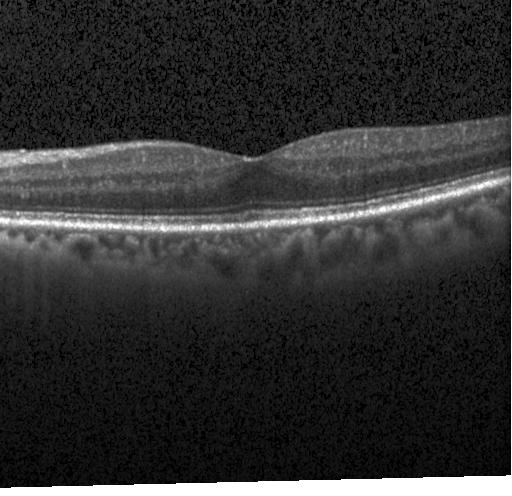

OCT B-scan. Fovea-centered
Diagnosis: no evidence of CNV, DME, or drusen.